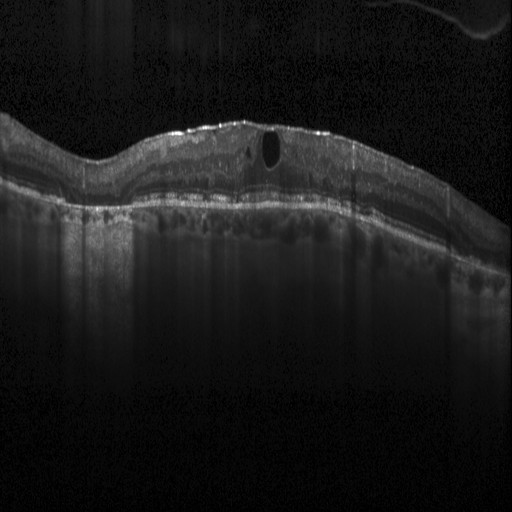

OCT B-scan; SD-OCT
Diagnosis: diabetic macular edema.